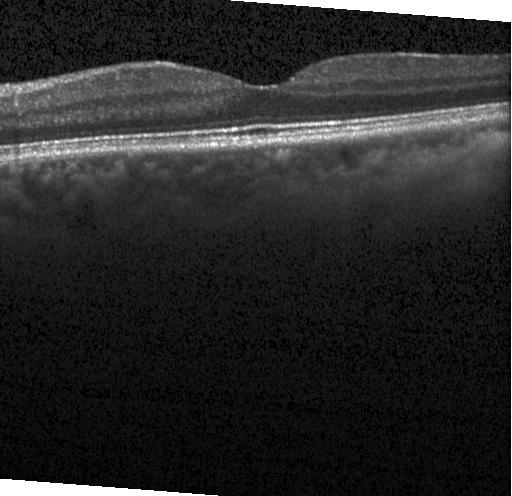 OCT line scan · horizontal scan through the fovea · Heidelberg Spectralis OCT system · spectral-domain OCT
OCT finding: no evidence of choroidal neovascularization, diabetic macular edema, or drusen.